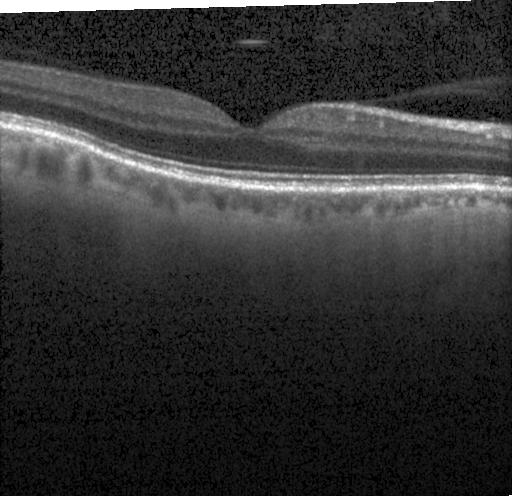

Neither choroidal neovascularization, diabetic macular edema, nor drusen.